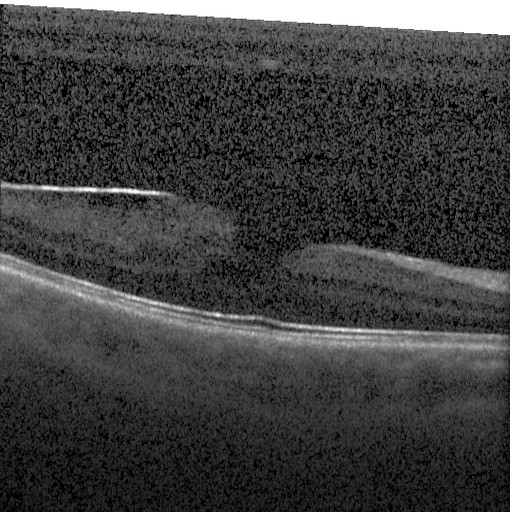 OCT line scan. Heidelberg Spectralis OCT system. Spectral-domain OCT. Impression: diabetic macular edema (DME).